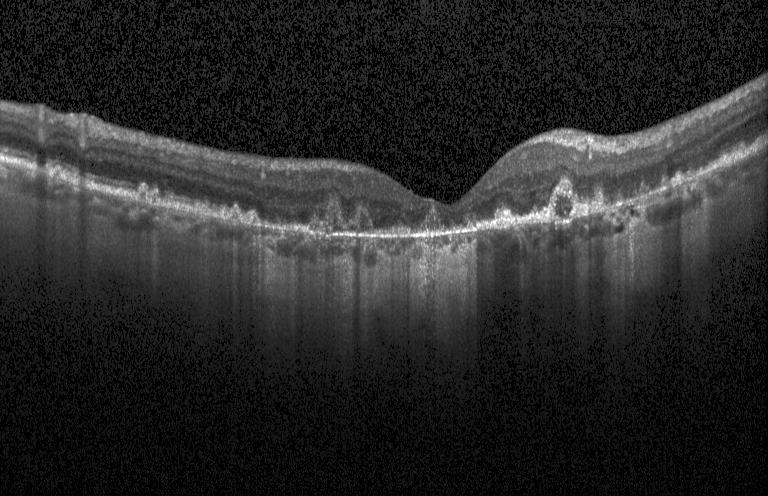
SD-OCT; retinal OCT B-scan
OCT finding: choroidal neovascularization.